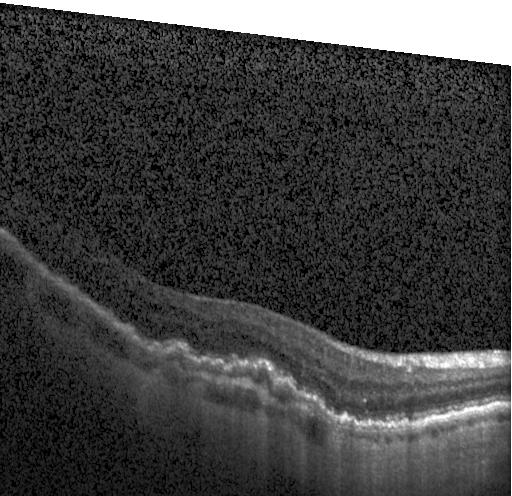

Spectral-domain optical coherence tomography · retinal OCT B-scan · Heidelberg Spectralis OCT system · fovea-centered. Diagnosis: CNV.